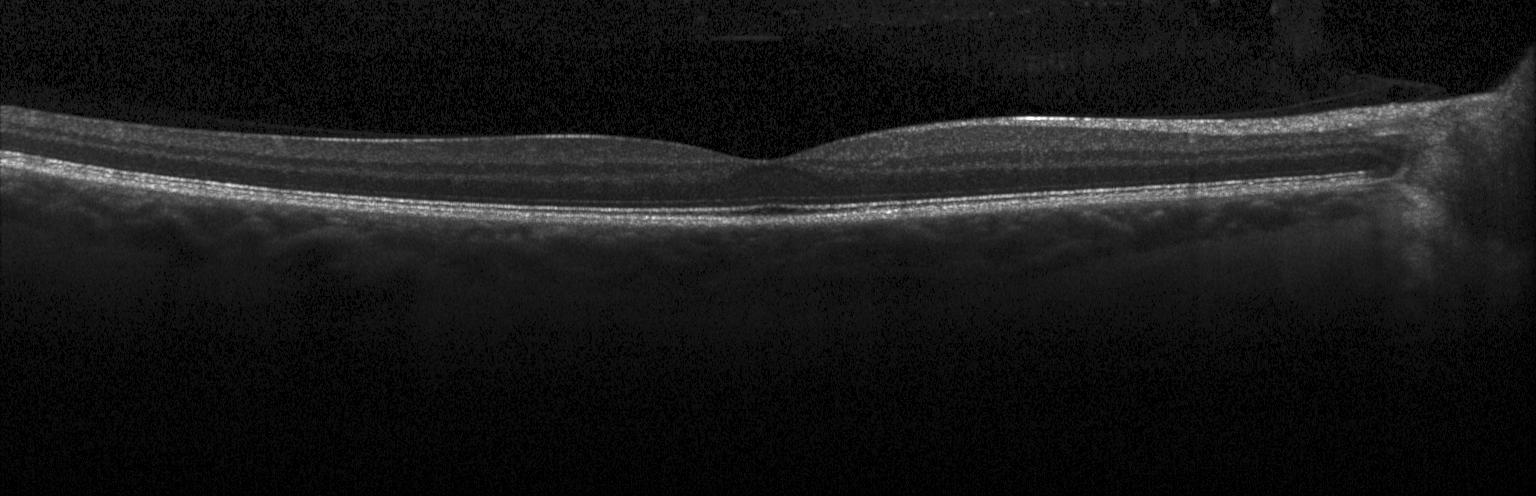
OCT line scan · Heidelberg Spectralis.
No choroidal neovascularization, no diabetic macular edema, and no drusen.